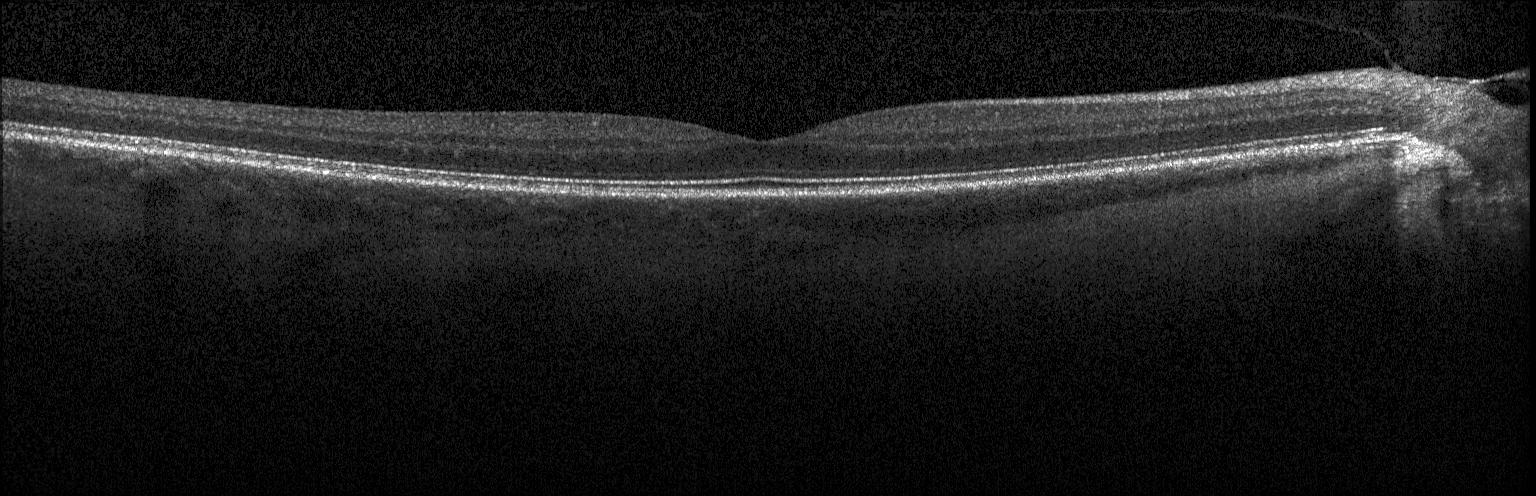 Spectral-domain optical coherence tomography; OCT line scan; macular scan
Diagnosis: no evidence of choroidal neovascularization, diabetic macular edema, or drusen.